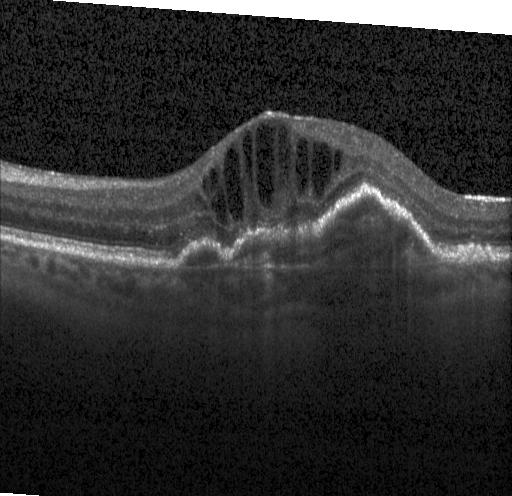 Impression: choroidal neovascularization.